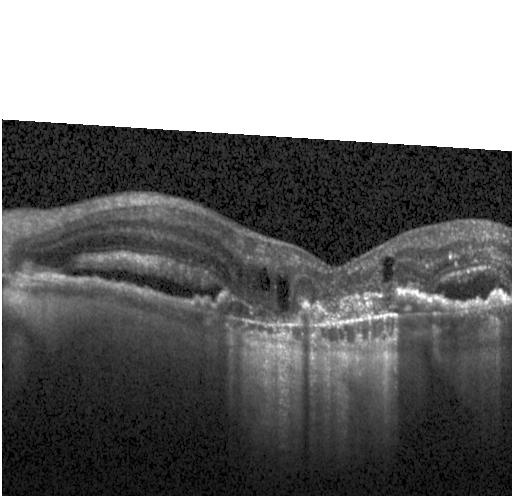

Assessment: a choroidal neovascular membrane.